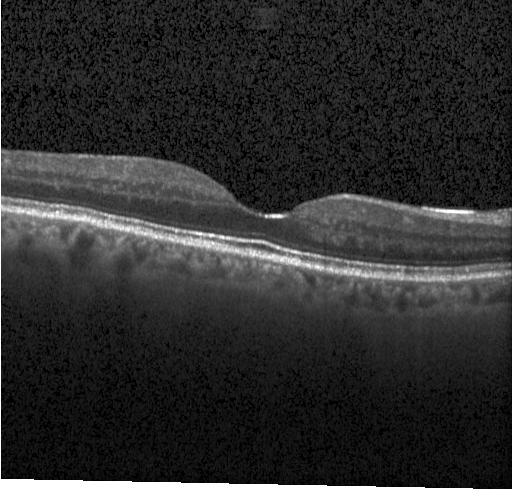

This B-scan demonstrates no evidence of choroidal neovascularization, diabetic macular edema, or drusen.